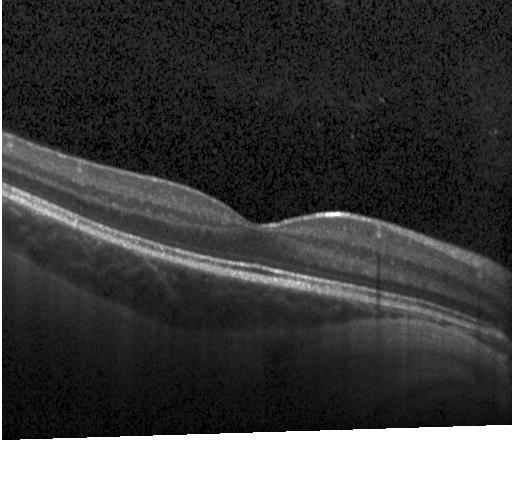

Macular OCT demonstrating neither choroidal neovascularization, diabetic macular edema, nor drusen.